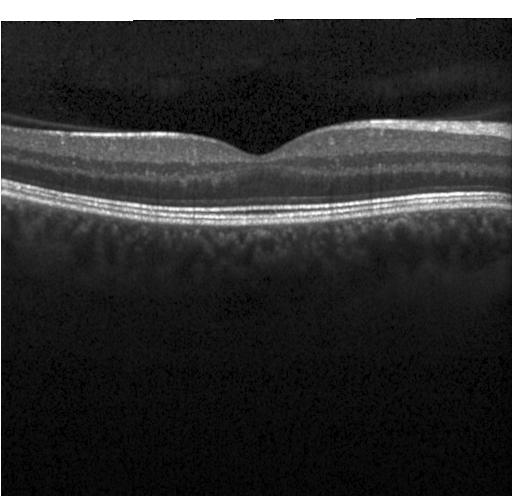
Retinal OCT cross-section.
Finding: no choroidal neovascularization, no diabetic macular edema, and no drusen.